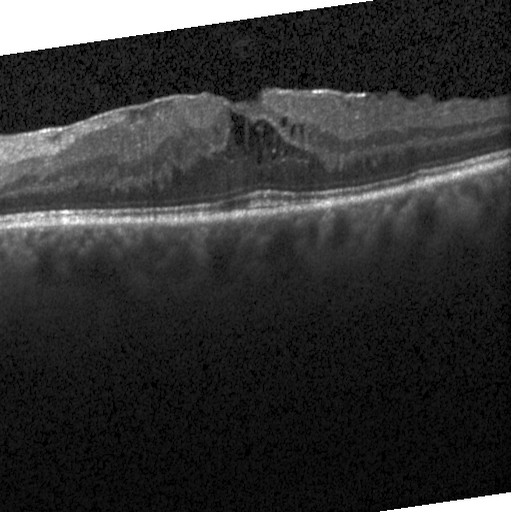 Acquired on a Heidelberg Spectralis; spectral-domain OCT; fovea-centered; OCT B-scan
Diagnosis: diabetic macular edema.